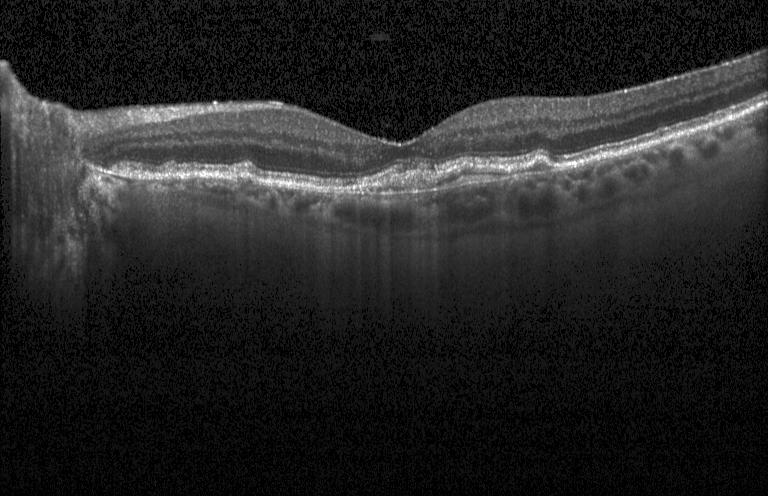
Impression: a choroidal neovascular membrane.